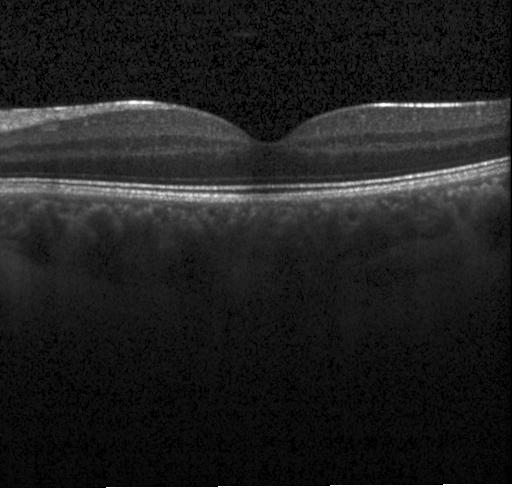

The scan shows no choroidal neovascularization, diabetic macular edema, or drusen.